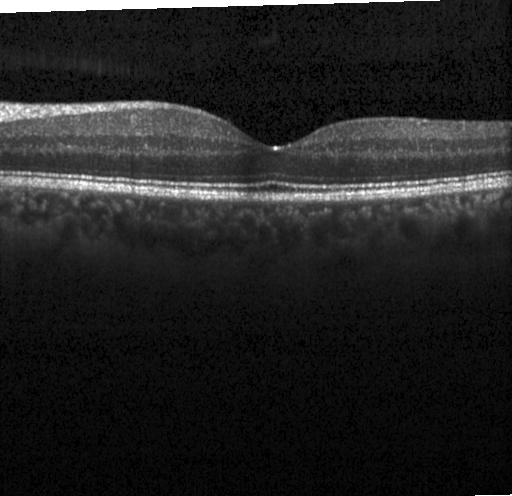

OCT line scan; macular scan; Heidelberg Spectralis OCT system
Diagnosis: no choroidal neovascularization, diabetic macular edema, or drusen.